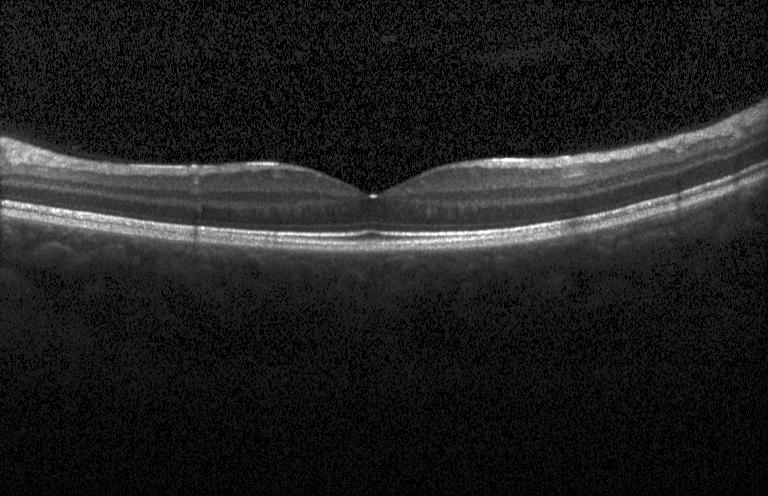

Retinal OCT cross-section showing no evidence of choroidal neovascularization, diabetic macular edema, or drusen.